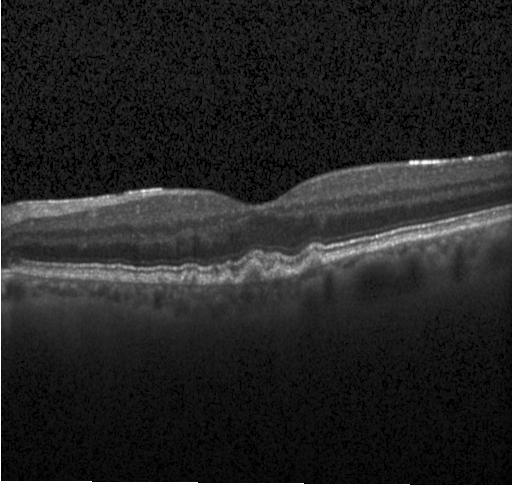

Retinal OCT cross-section, Heidelberg Spectralis OCT system, SD-OCT — Assessment: drusen.